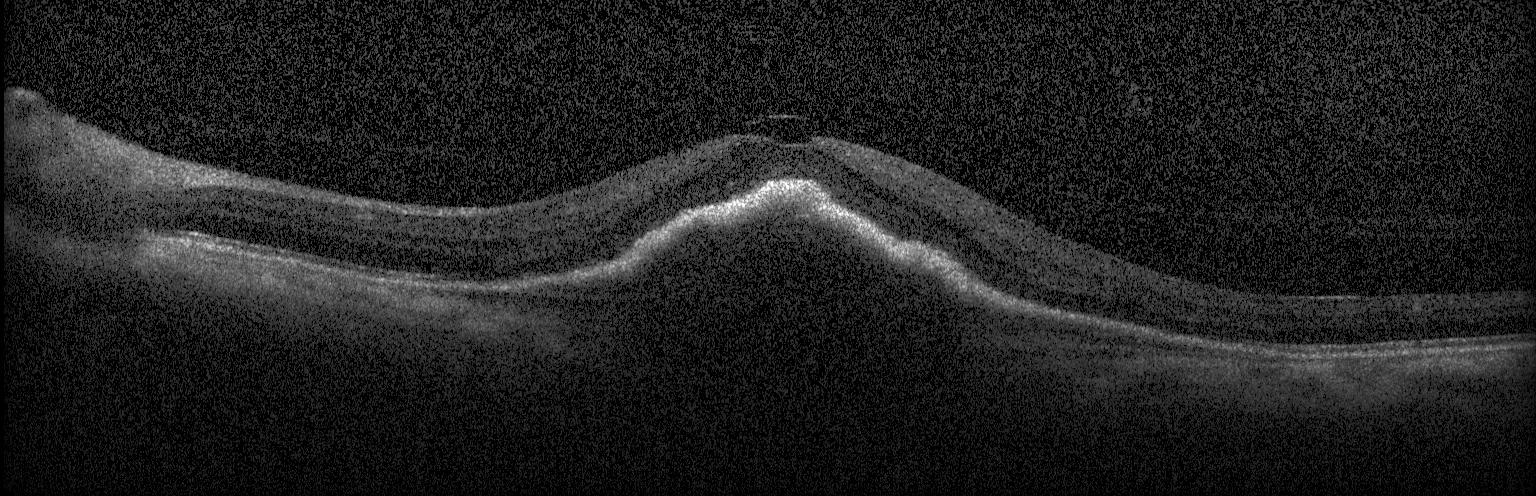

SD-OCT. OCT B-scan. Diagnosis: choroidal neovascularization (CNV).